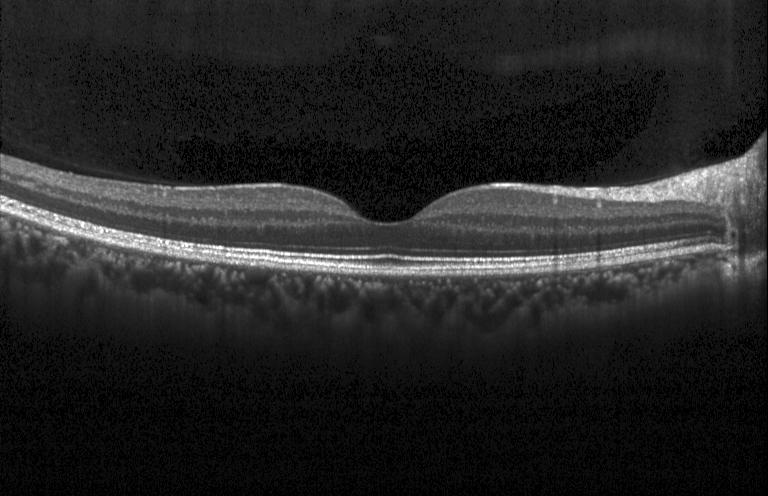

This B-scan demonstrates neither choroidal neovascularization, diabetic macular edema, nor drusen.